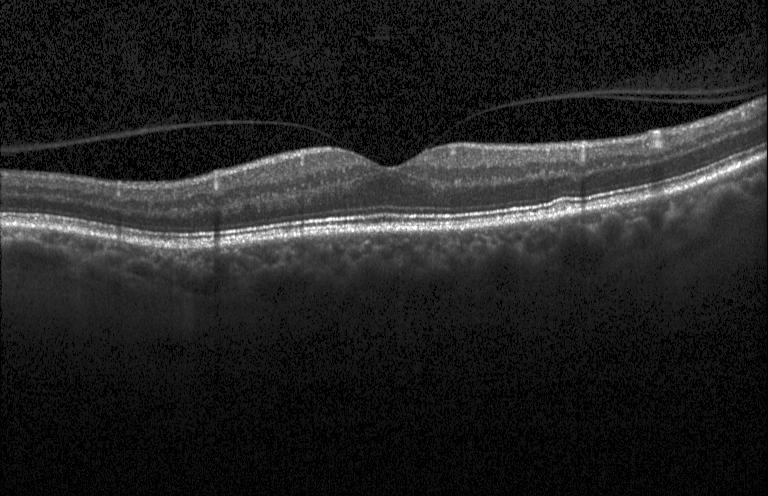 Retinal OCT B-scan, spectral-domain OCT
No evidence of choroidal neovascularization, diabetic macular edema, or drusen.